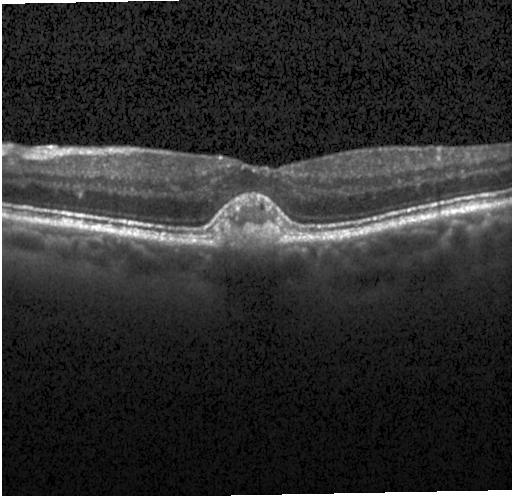

OCT finding: CNV.